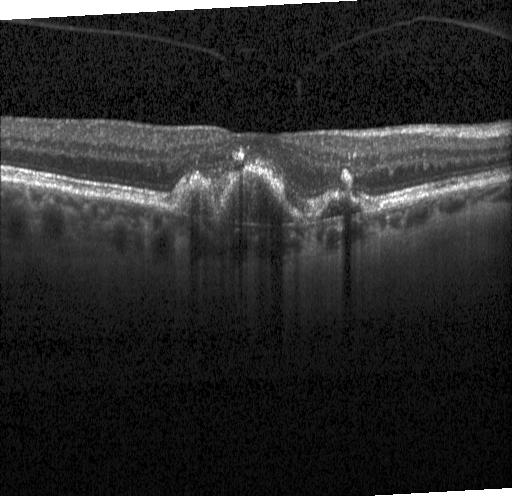
Retinal OCT cross-section; SD-OCT; fovea-centered
Impression: a choroidal neovascular membrane.